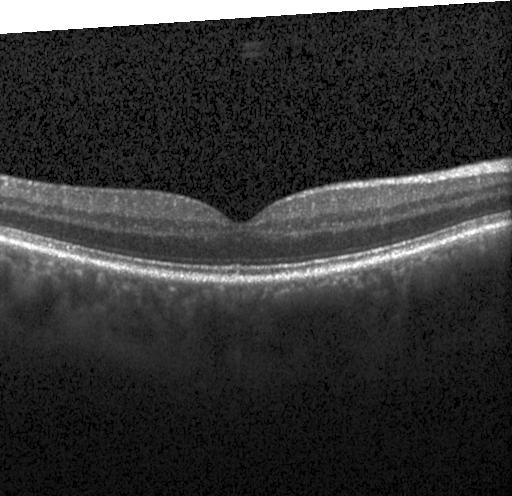 Dx: no choroidal neovascularization, diabetic macular edema, or drusen.